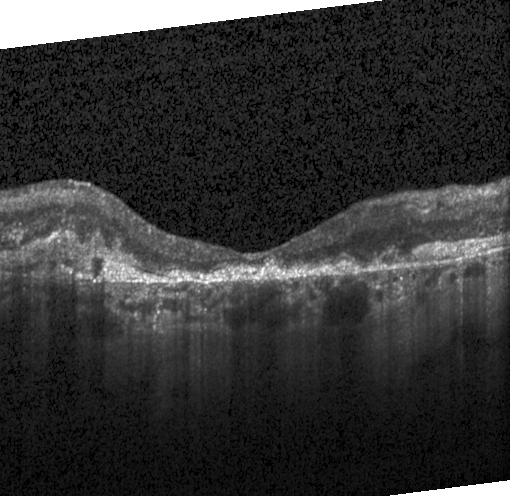 OCT B-scan; spectral-domain OCT; Heidelberg Spectralis
This B-scan demonstrates CNV.